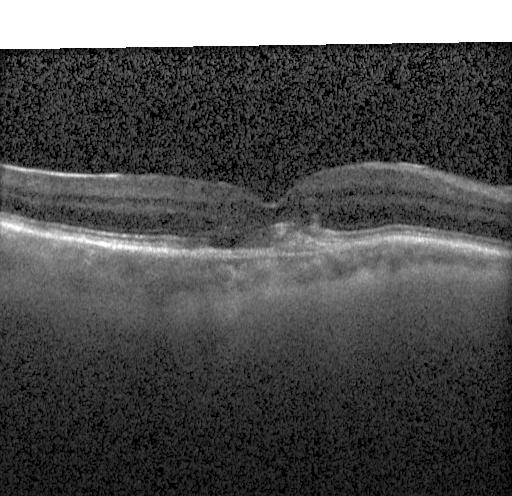
Optical coherence tomography scan; fovea-centered; Heidelberg Spectralis OCT system. Impression: a choroidal neovascular membrane.